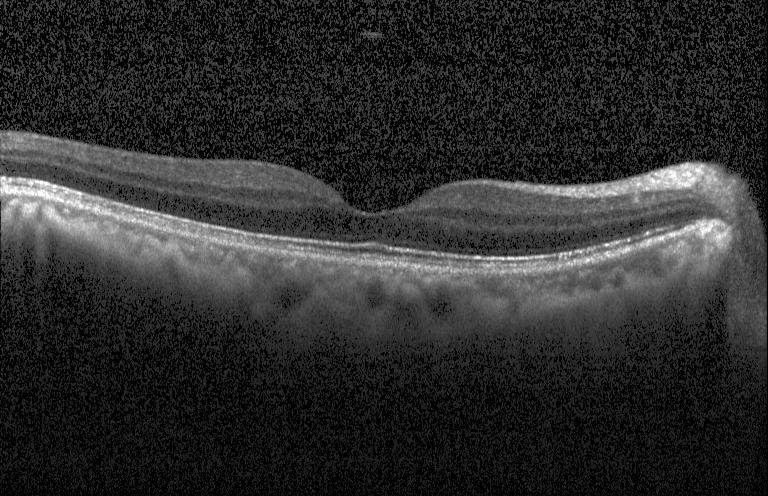
OCT B-scan — This B-scan demonstrates no CNV, no DME, and no drusen.